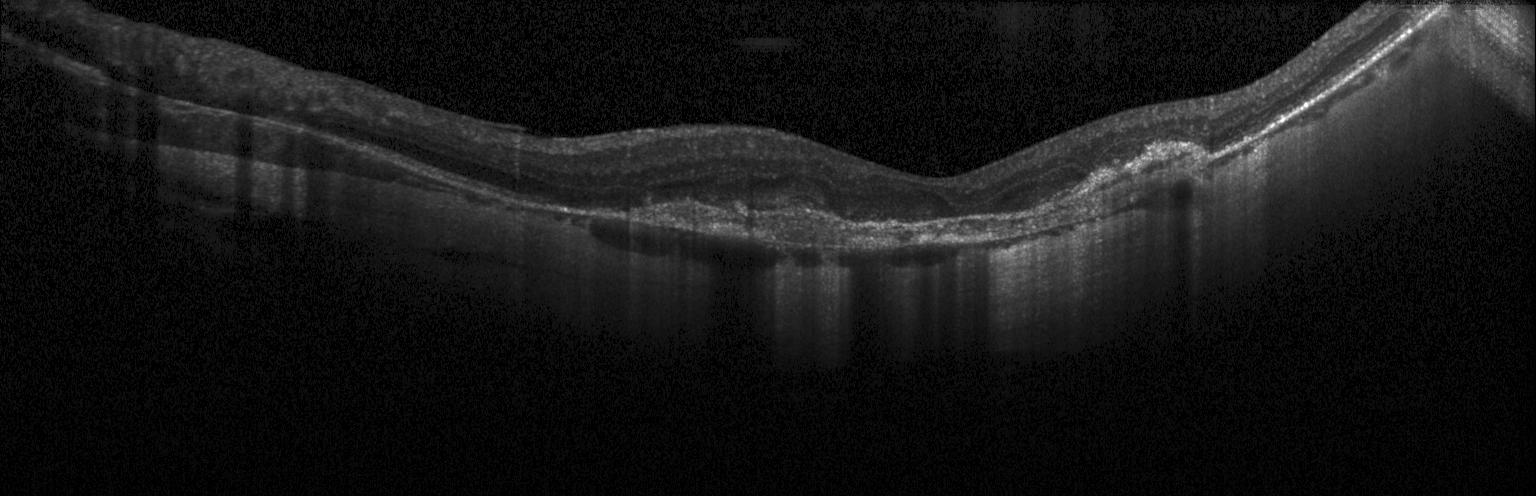

SD-OCT; optical coherence tomography B-scan — Finding: a choroidal neovascular membrane.